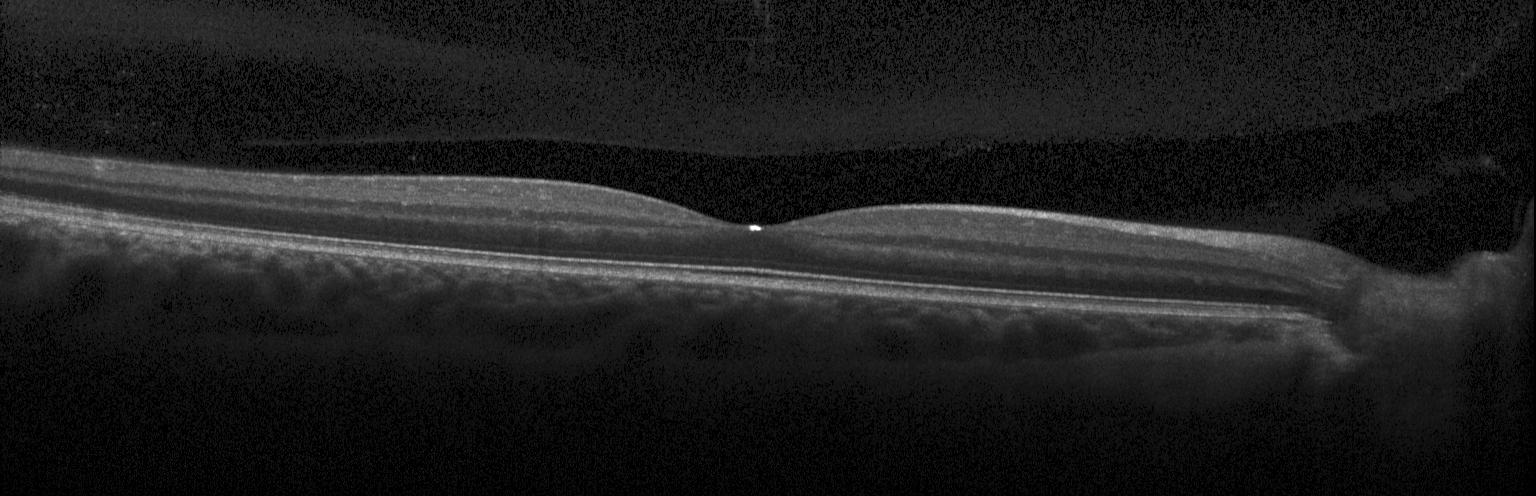 Optical coherence tomography scan; horizontal scan through the fovea. The scan shows no choroidal neovascularization, diabetic macular edema, or drusen.